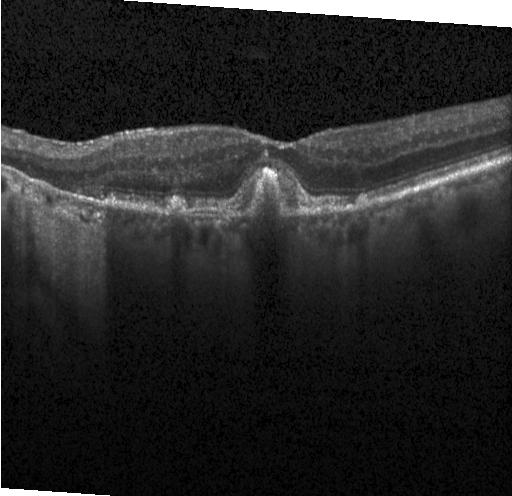
Fovea-centered; optical coherence tomography scan; spectral-domain optical coherence tomography. OCT finding: CNV.